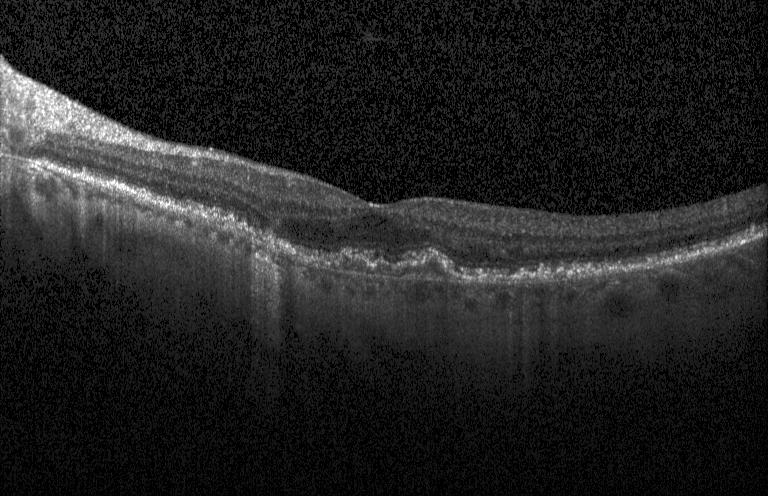 OCT B-scan.
A choroidal neovascular membrane.